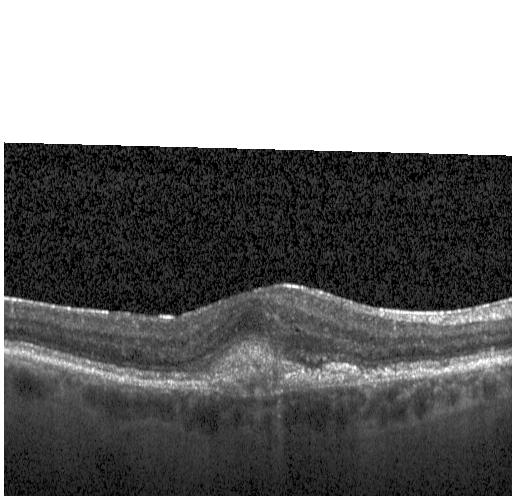
Horizontal scan through the fovea · OCT line scan · spectral-domain optical coherence tomography
Finding: choroidal neovascularization.